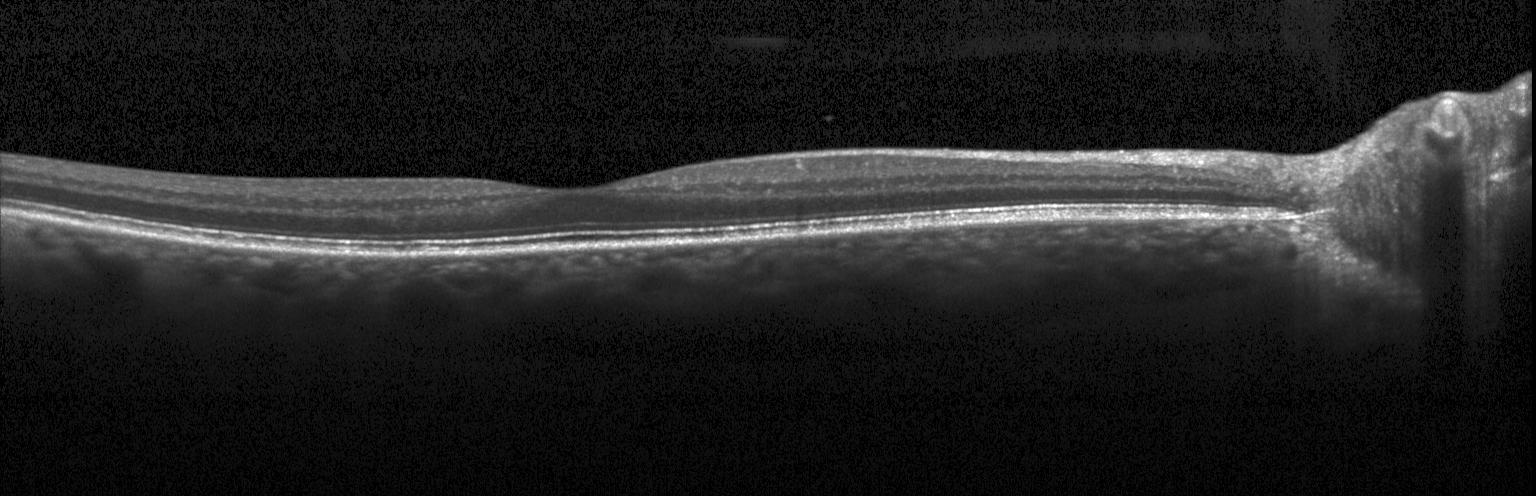
Horizontal scan through the fovea · spectral-domain optical coherence tomography · Heidelberg Spectralis · retinal OCT cross-section. Diagnosis: no CNV, DME, or drusen.